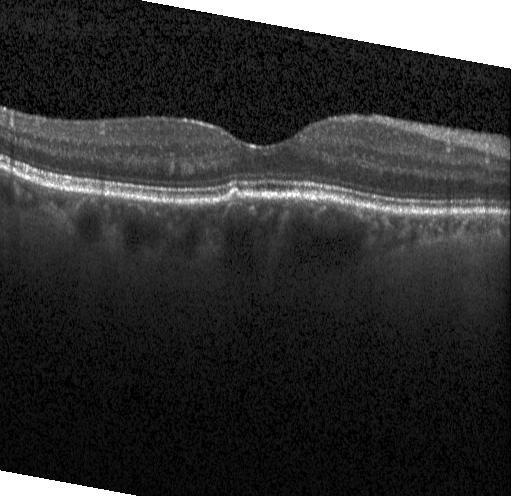

SD-OCT; optical coherence tomography B-scan — Diagnosis: multiple drusen.